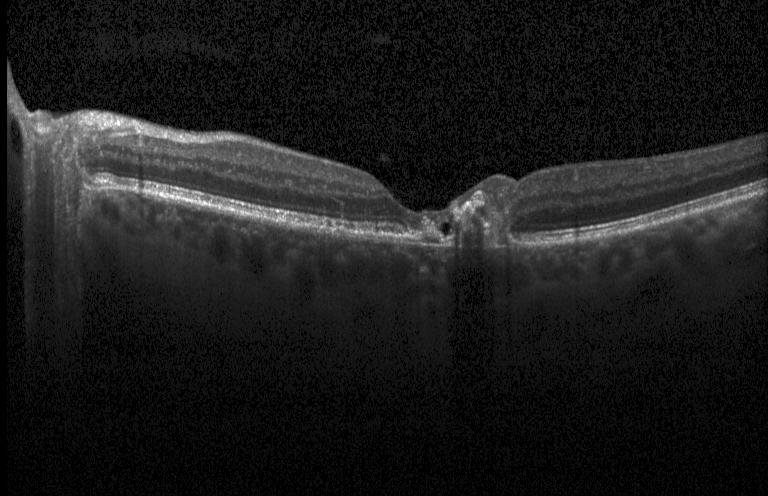

OCT line scan, through the macula, Heidelberg Spectralis, spectral-domain optical coherence tomography. Dx: a choroidal neovascular membrane.